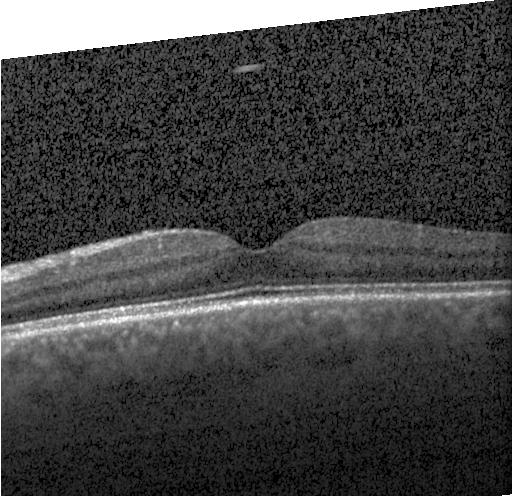 Heidelberg Spectralis, spectral-domain OCT, fovea-centered, optical coherence tomography scan. Macular OCT: no choroidal neovascularization, diabetic macular edema, or drusen.